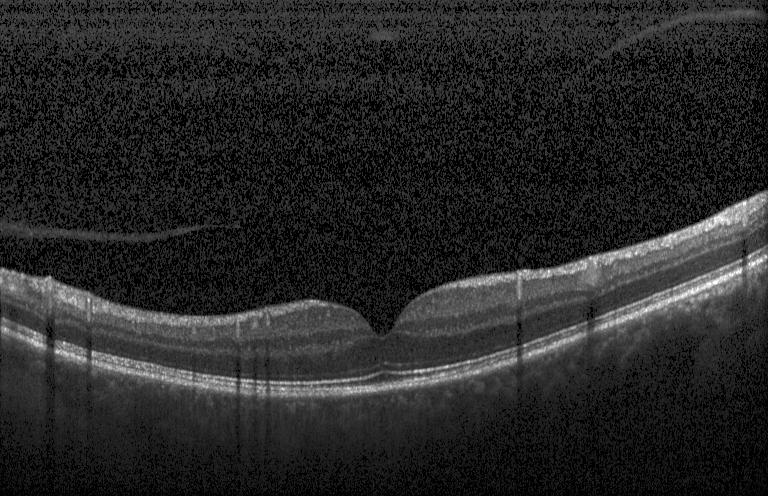

Macular OCT: neither CNV, DME, nor drusen.